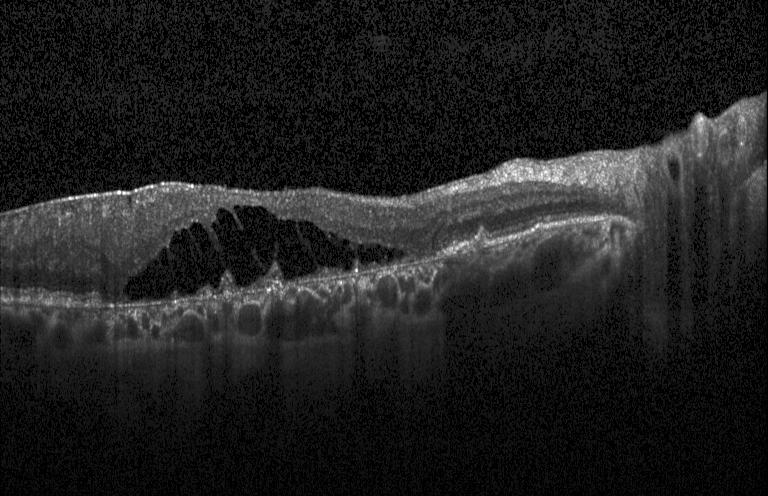

Instrument: Heidelberg Spectralis; macular scan; OCT line scan; spectral-domain OCT
Dx: choroidal neovascularization (CNV).